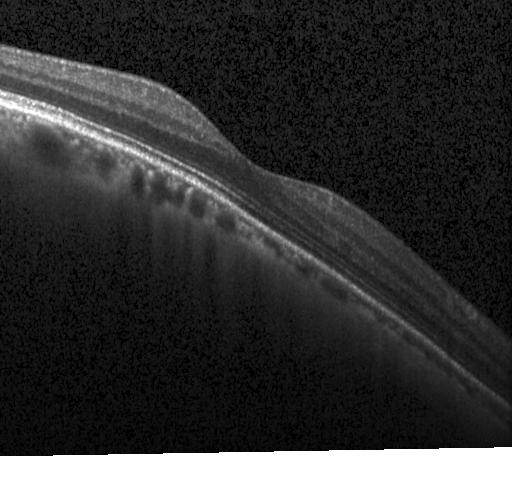

OCT scan showing no choroidal neovascularization, diabetic macular edema, or drusen.